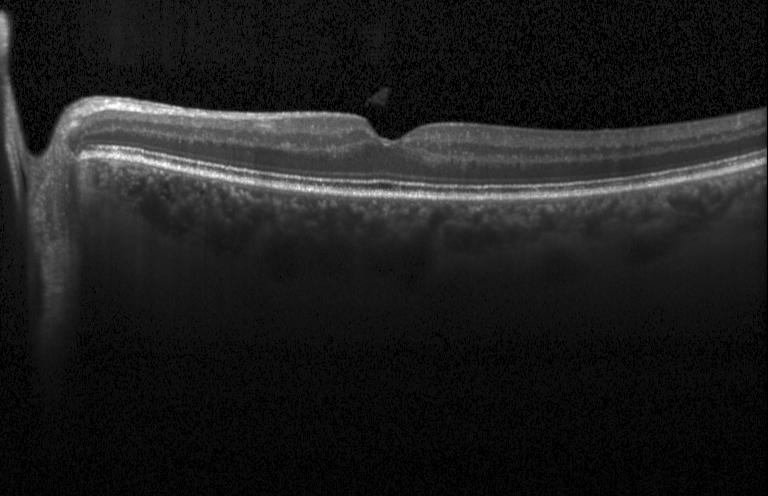
Spectral-domain OCT, through the macula, retinal OCT B-scan, instrument: Heidelberg Spectralis — Impression: no choroidal neovascularization, diabetic macular edema, or drusen.